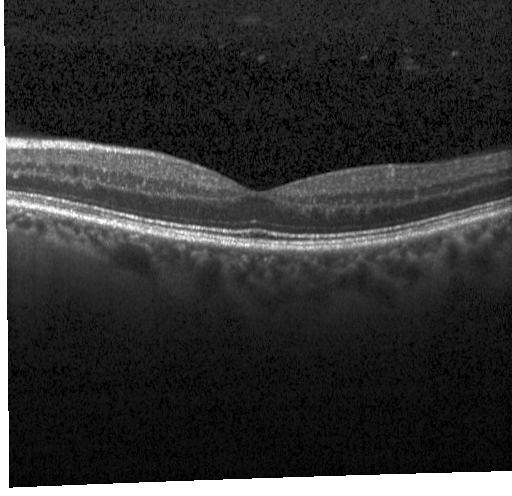
This B-scan demonstrates no choroidal neovascularization, diabetic macular edema, or drusen.